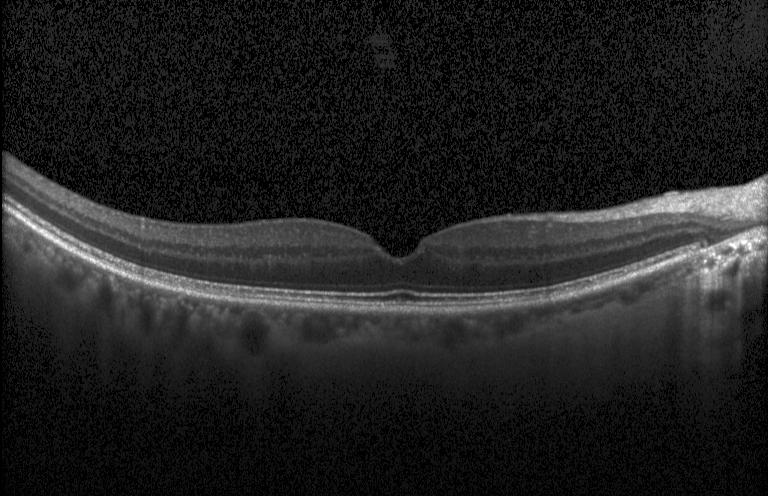 Heidelberg Spectralis, OCT line scan
No CNV, no DME, and no drusen.